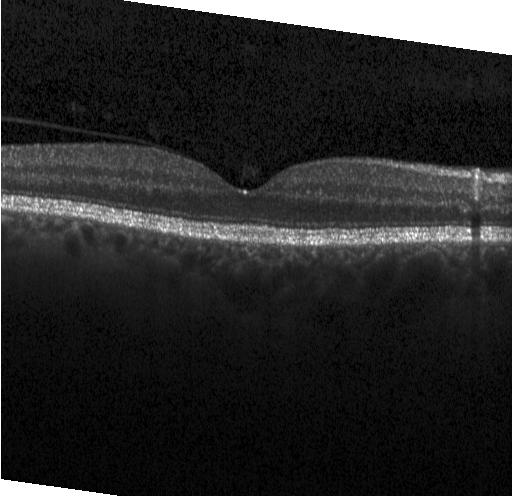
Assessment: neither choroidal neovascularization, diabetic macular edema, nor drusen.